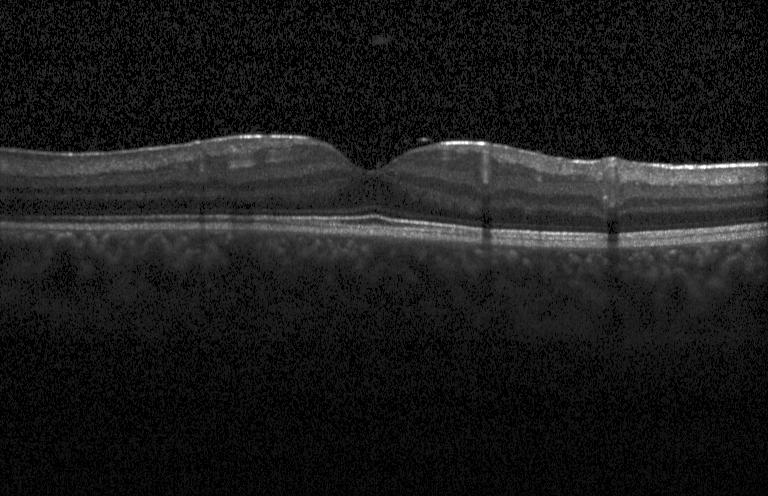

Instrument: Heidelberg Spectralis, optical coherence tomography B-scan, spectral-domain optical coherence tomography, through the macula — The scan shows no CNV, no DME, and no drusen.